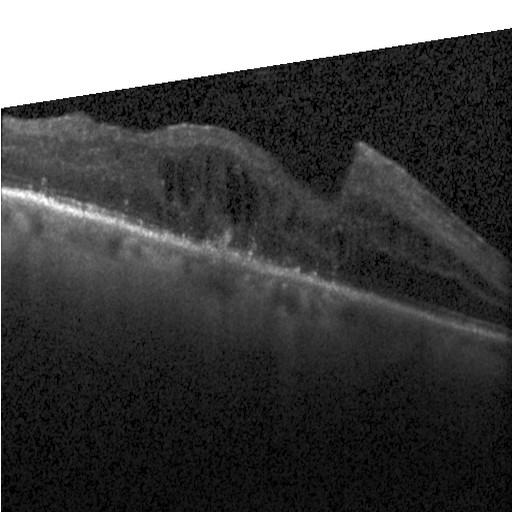
Spectral-domain OCT B-scan: diabetic macular edema (DME).